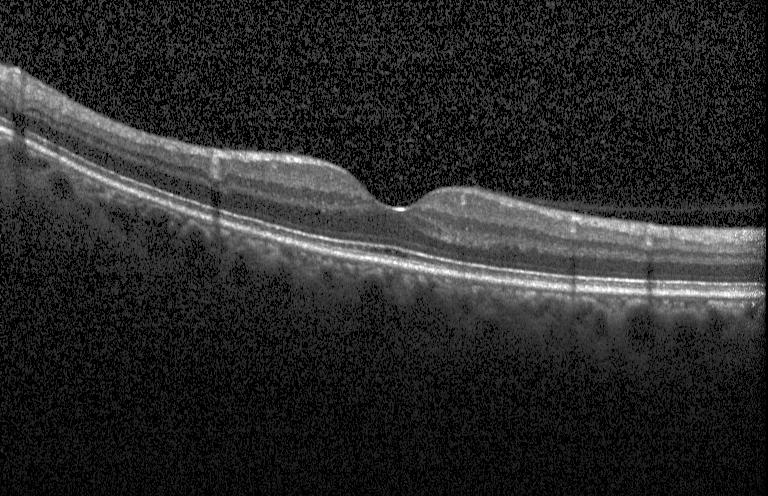 OCT B-scan; SD-OCT; Heidelberg Spectralis; horizontal scan through the fovea — OCT finding: no choroidal neovascularization, diabetic macular edema, or drusen.